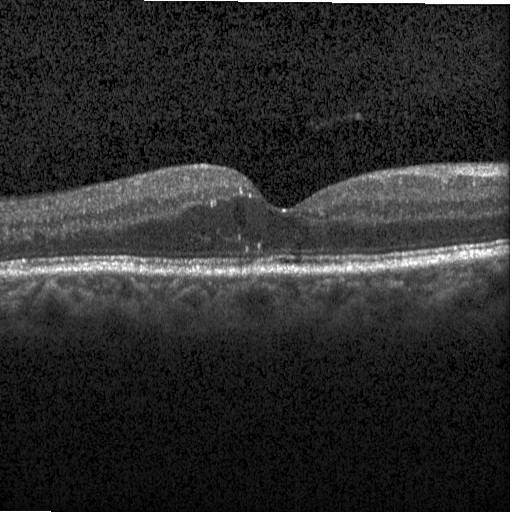 Retinal OCT B-scan; spectral-domain OCT.
Diagnosis: diabetic macular edema (DME).